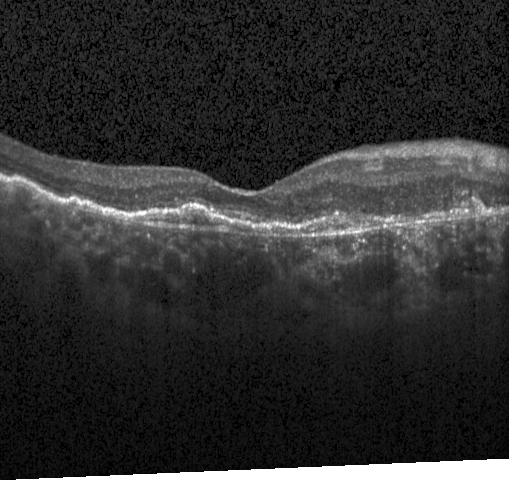

This B-scan demonstrates CNV.